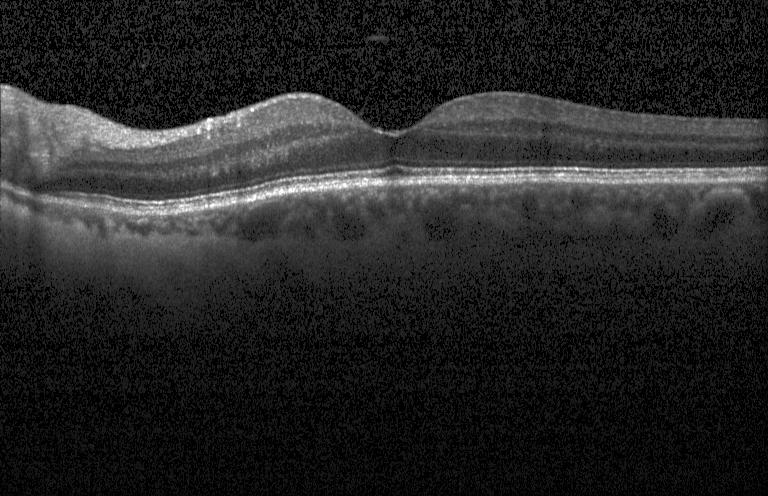

Impression: no choroidal neovascularization, diabetic macular edema, or drusen.